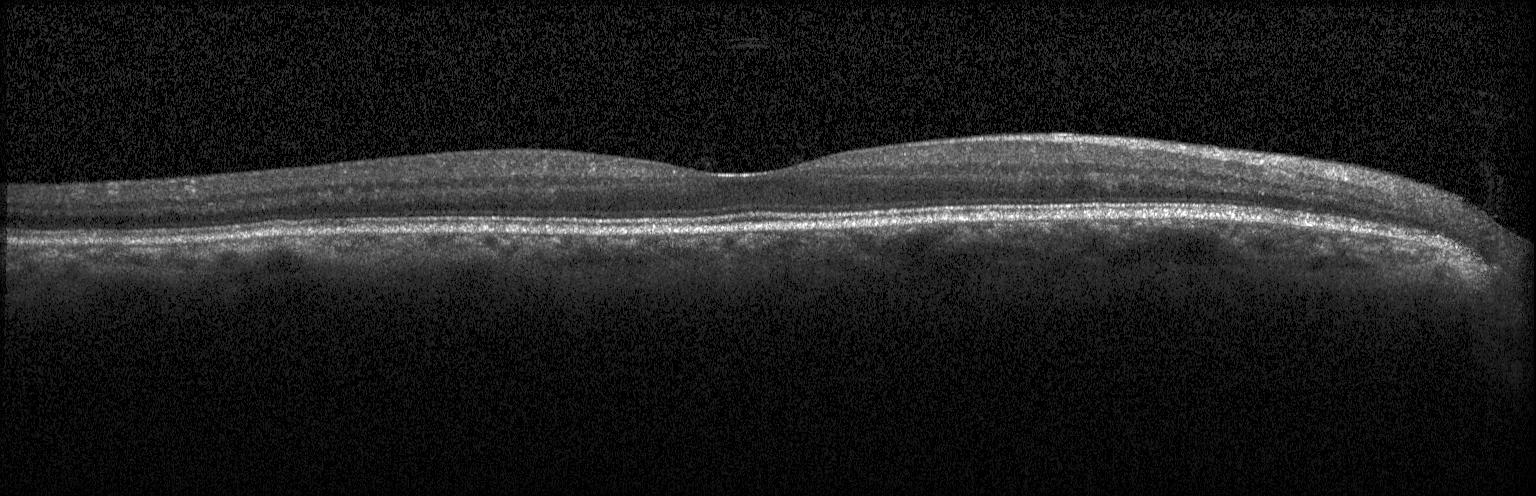
No choroidal neovascularization, diabetic macular edema, or drusen.